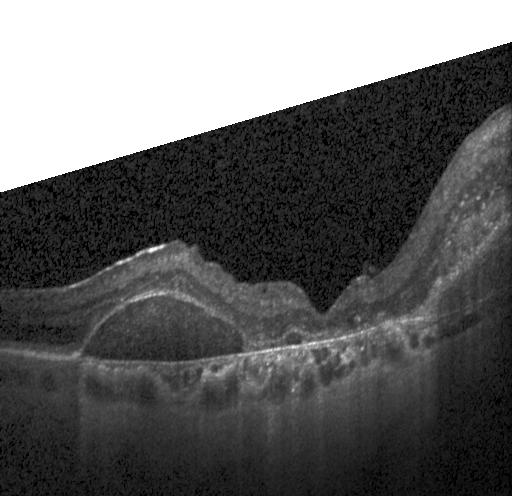
Instrument: Heidelberg Spectralis, SD-OCT, optical coherence tomography scan
A choroidal neovascular membrane.